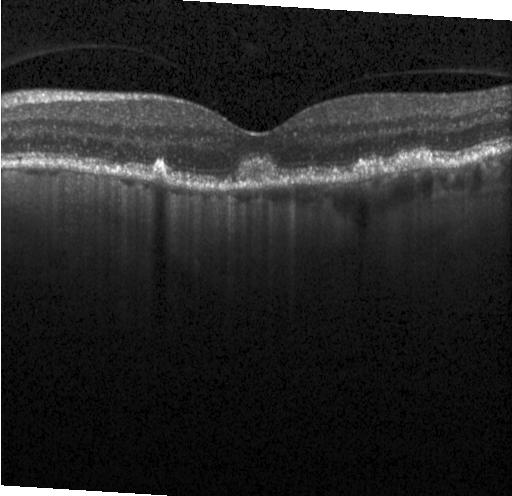 Centered on the fovea, retinal OCT cross-section — Impression: multiple drusen.